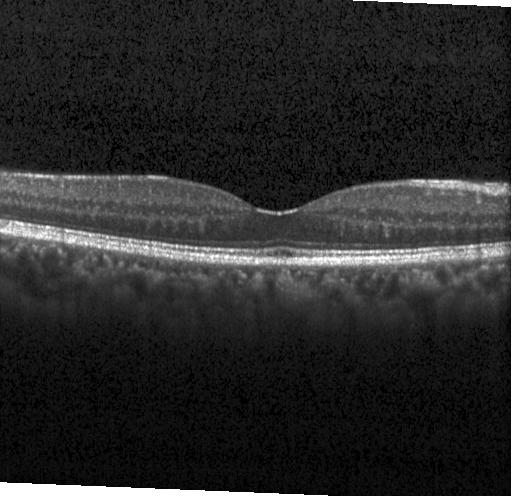

Diagnosis: neither choroidal neovascularization, diabetic macular edema, nor drusen.